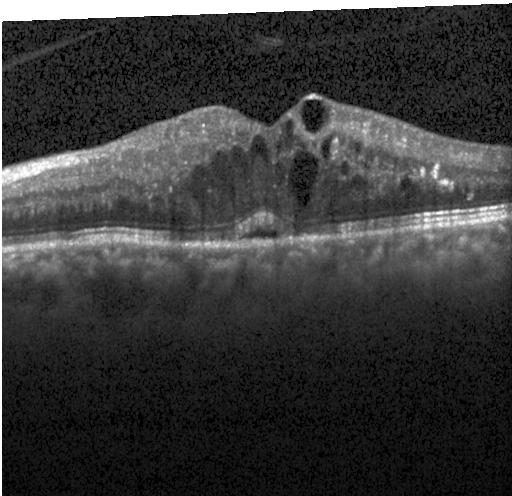 Optical coherence tomography B-scan; spectral-domain optical coherence tomography; instrument: Heidelberg Spectralis — Diabetic macular edema (DME).